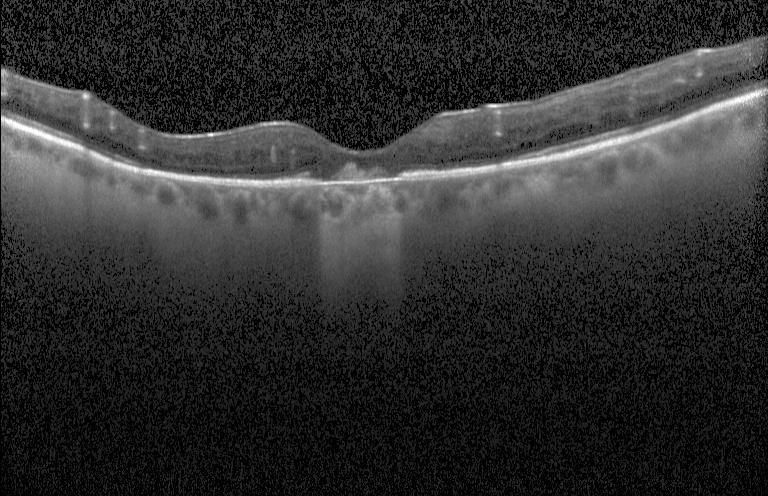
Optical coherence tomography scan; Heidelberg Spectralis; spectral-domain OCT
Macular OCT: a choroidal neovascular membrane.